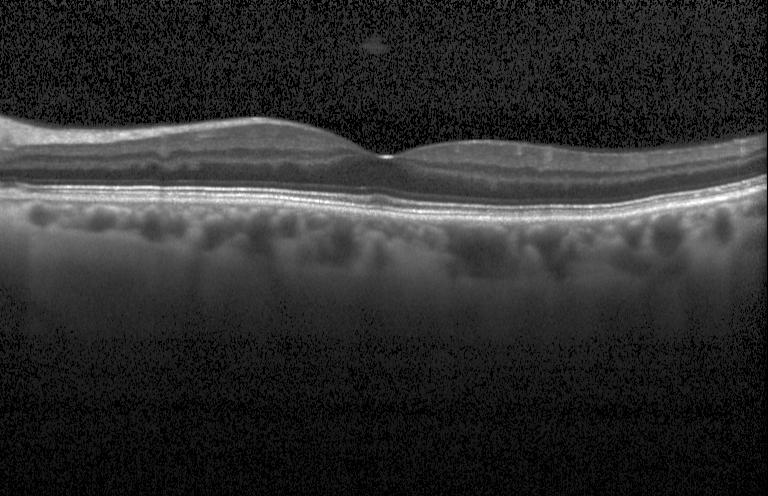
This B-scan demonstrates no evidence of choroidal neovascularization, diabetic macular edema, or drusen.